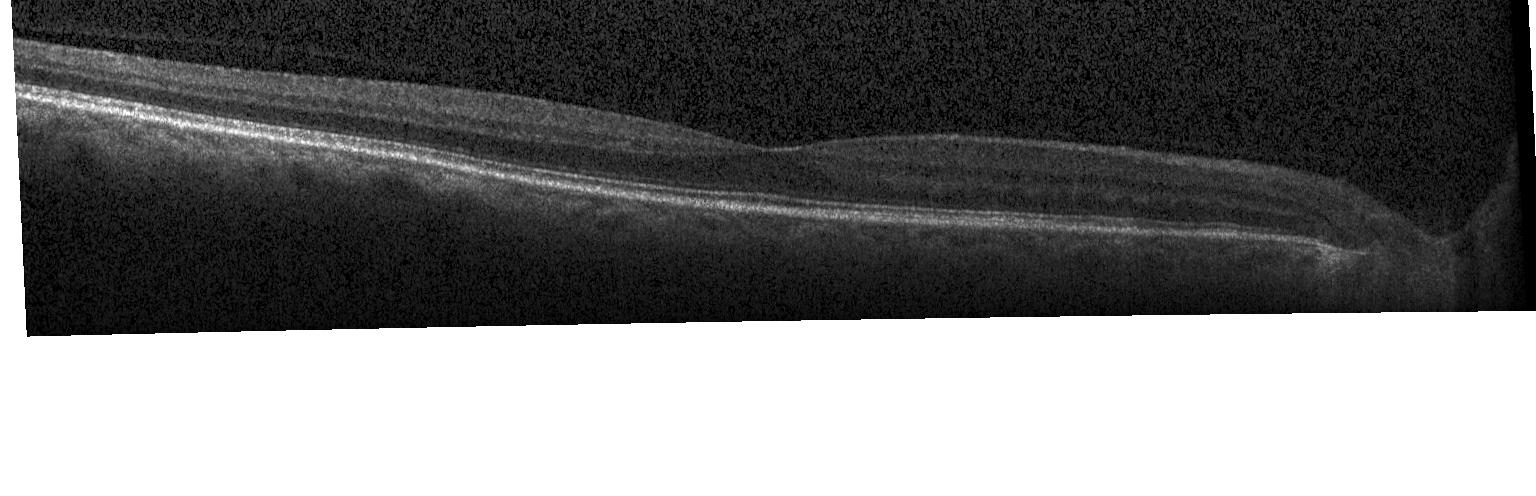

OCT line scan; Heidelberg Spectralis OCT system. Assessment: neither CNV, DME, nor drusen.